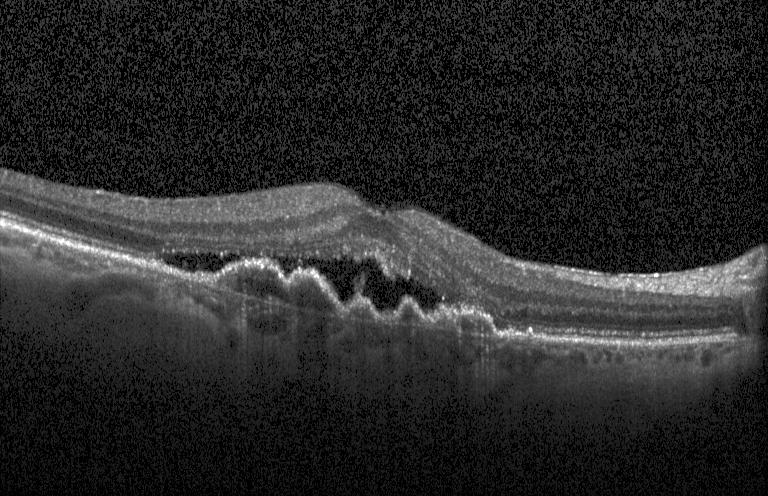

Retinal OCT cross-section showing a choroidal neovascular membrane.